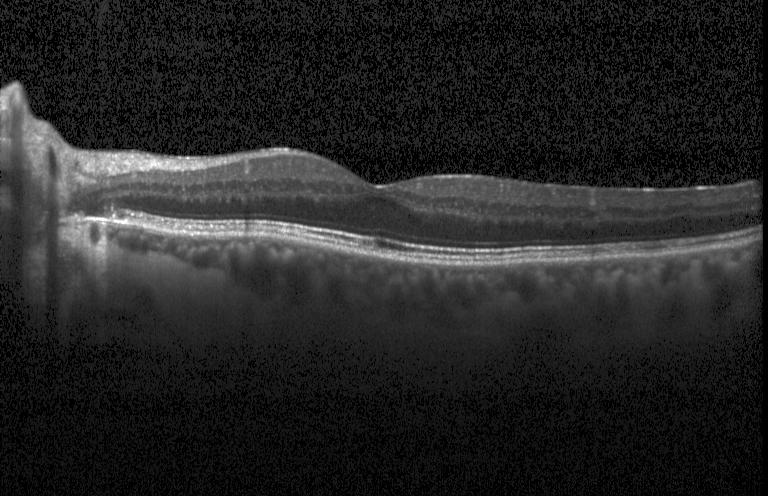

This B-scan demonstrates no evidence of choroidal neovascularization, diabetic macular edema, or drusen.